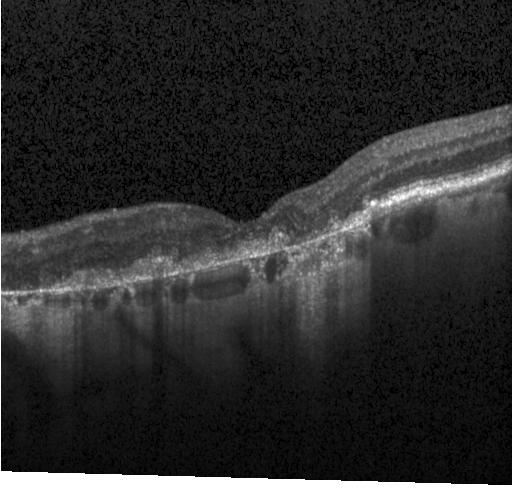
Optical coherence tomography B-scan
OCT finding: CNV.